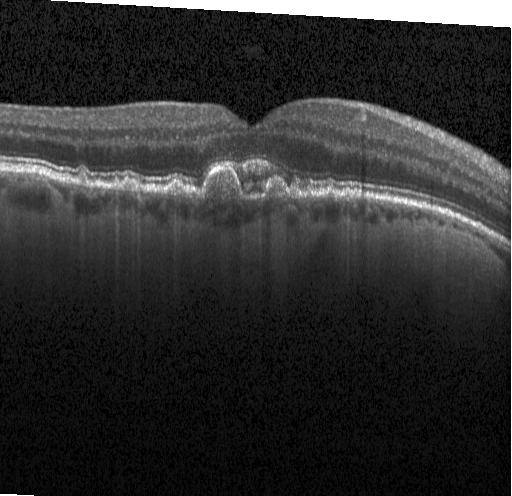
Heidelberg Spectralis OCT system; retinal OCT cross-section; SD-OCT
Impression: multiple drusen.